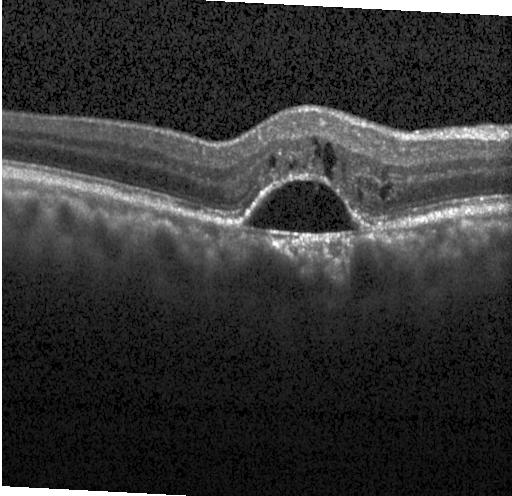

Acquired on a Heidelberg Spectralis, retinal OCT B-scan.
Assessment: a choroidal neovascular membrane.